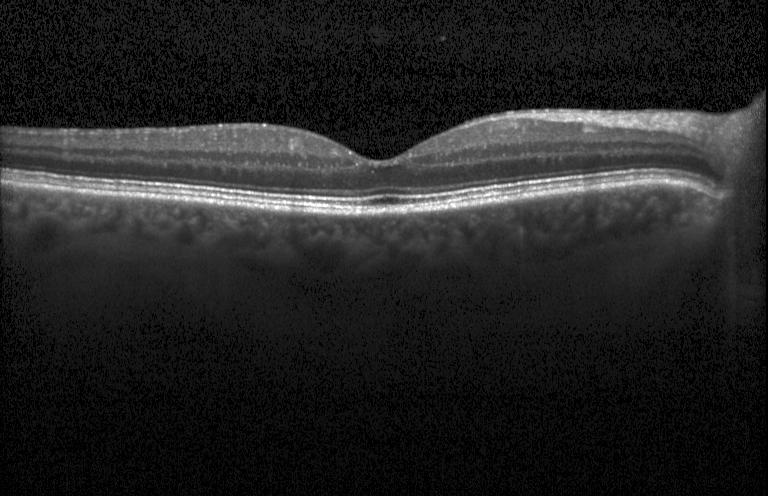 Neither choroidal neovascularization, diabetic macular edema, nor drusen.